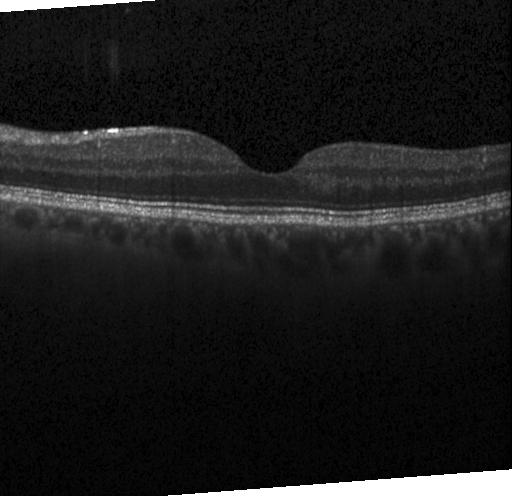
OCT B-scan · instrument: Heidelberg Spectralis.
Diagnosis: no CNV, DME, or drusen.